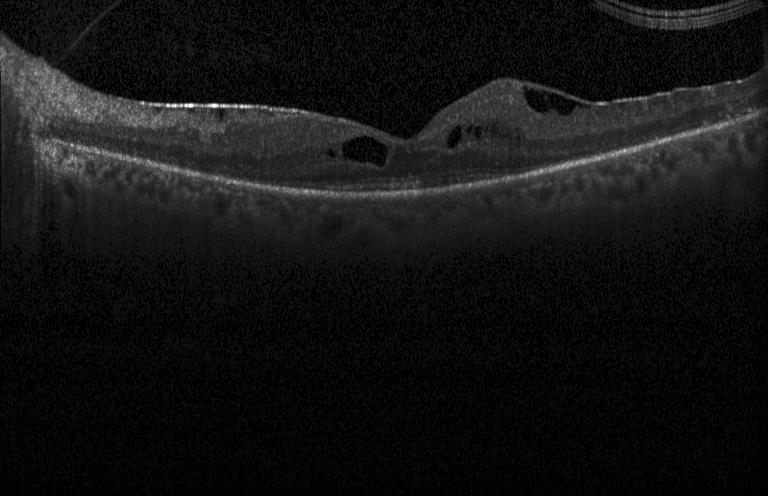

Impression: diabetic macular edema (DME).